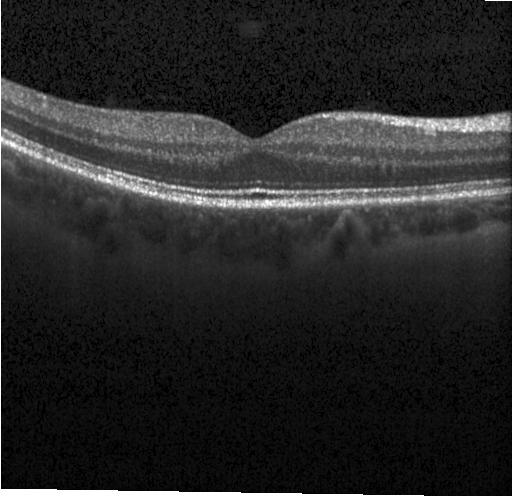

OCT line scan. Spectral-domain OCT. Horizontal scan through the fovea.
This B-scan demonstrates no choroidal neovascularization, diabetic macular edema, or drusen.